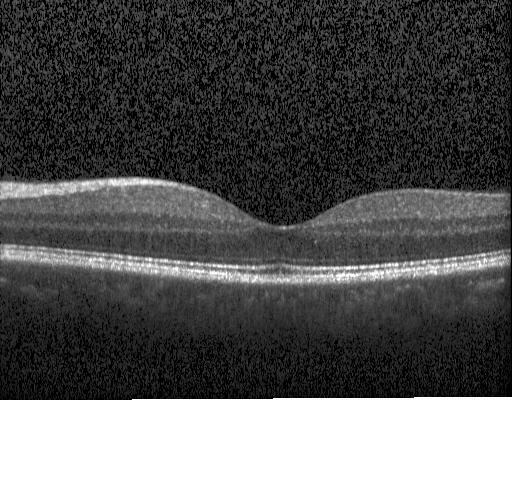 Spectral-domain OCT B-scan: no choroidal neovascularization, no diabetic macular edema, and no drusen.